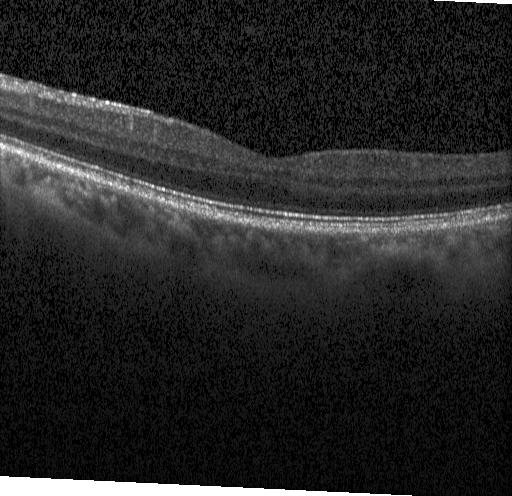
The scan shows no CNV, no DME, and no drusen.